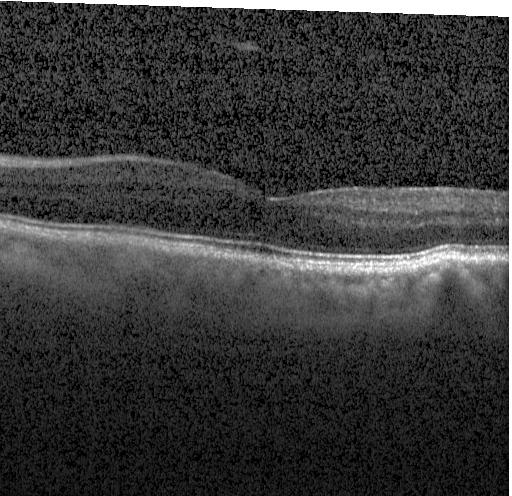 Fovea-centered · optical coherence tomography scan — Finding: no choroidal neovascularization, no diabetic macular edema, and no drusen.